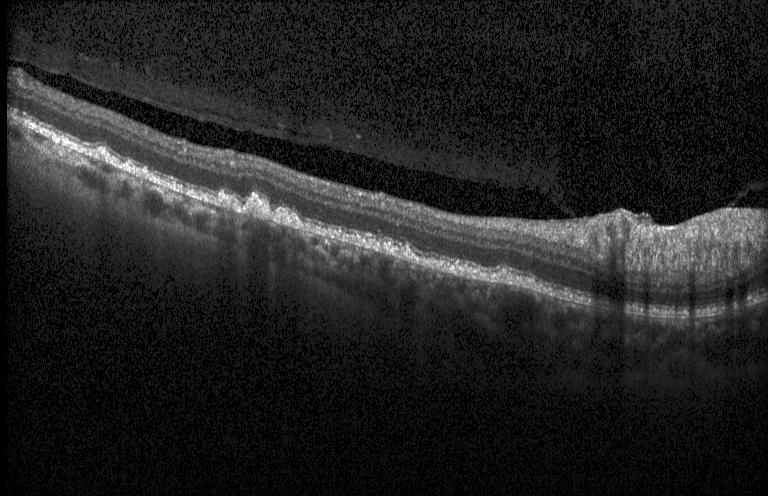 OCT finding: drusen.